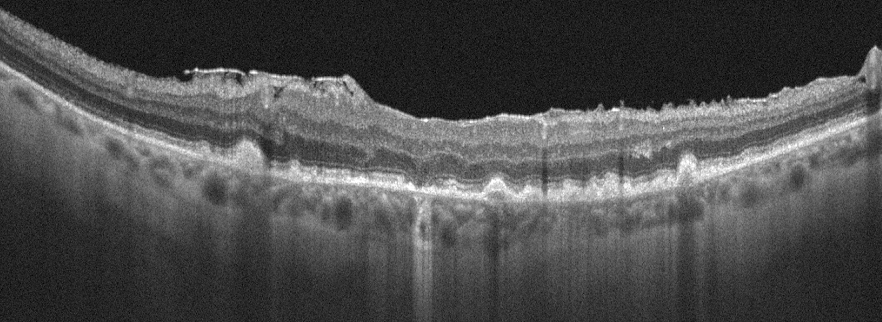
Right eye; OCT B-scan.
Finding: AMD.